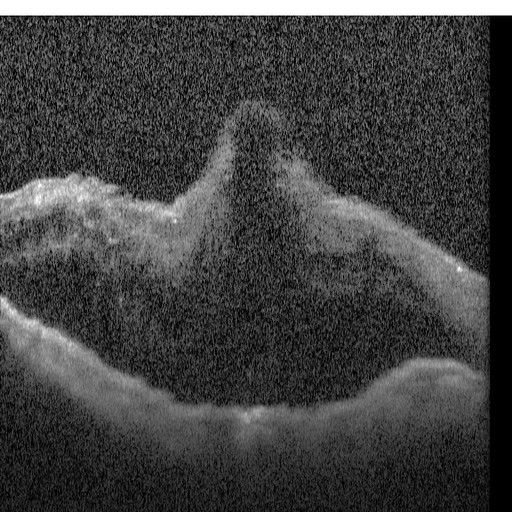 OCT scan showing DME.